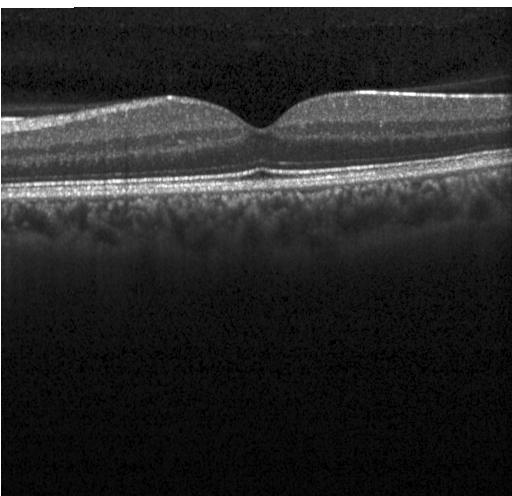
SD-OCT · acquired on a Heidelberg Spectralis · macular scan · OCT line scan — This B-scan demonstrates neither choroidal neovascularization, diabetic macular edema, nor drusen.